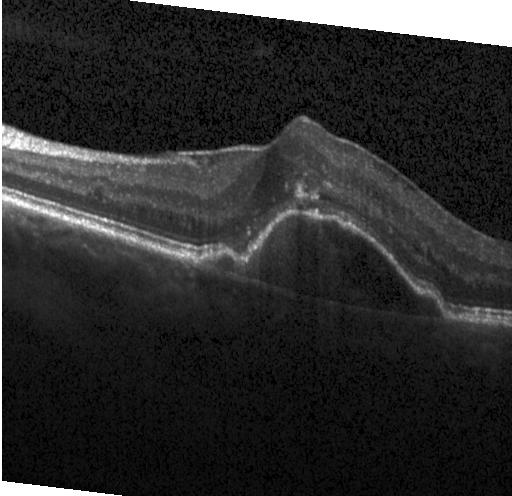

Diagnosis: choroidal neovascularization.